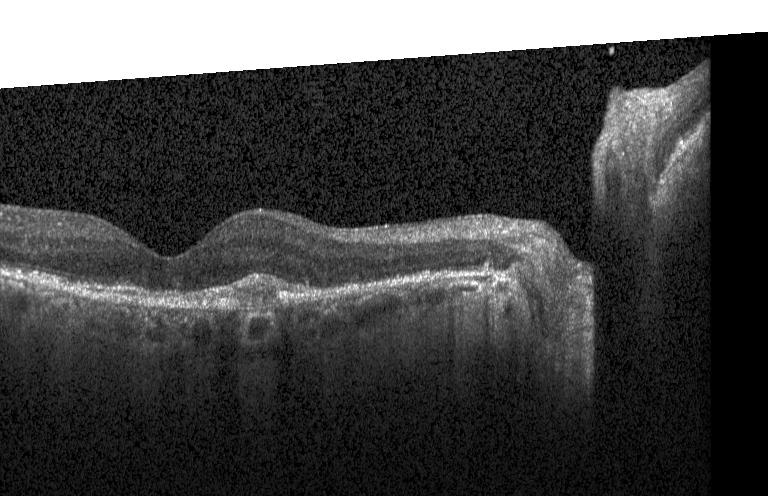 OCT line scan.
Impression: CNV.